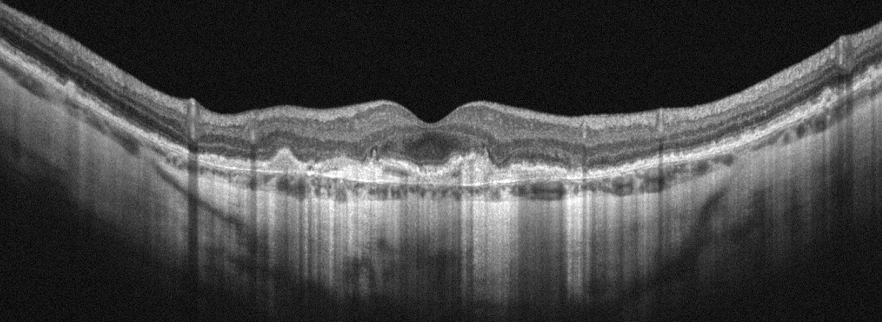 Retinal OCT cross-section — Impression: AMD.